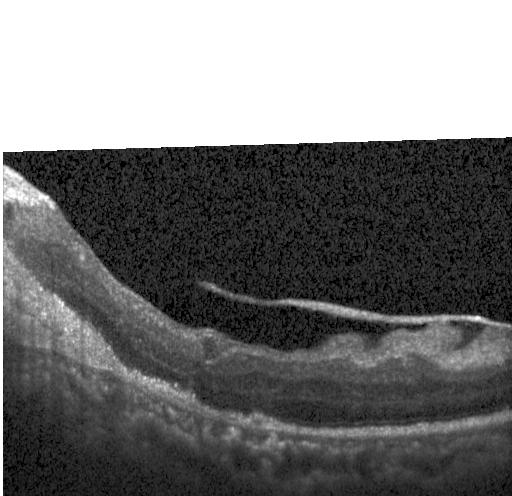 Diagnosis: a choroidal neovascular membrane.